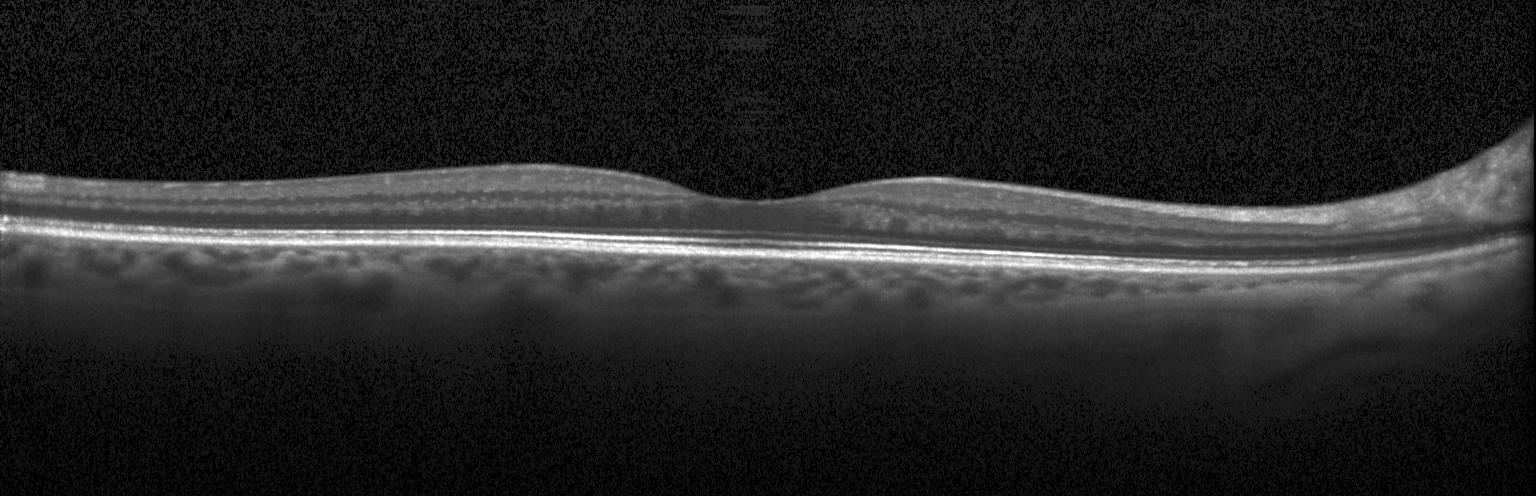

OCT B-scan showing no evidence of choroidal neovascularization, diabetic macular edema, or drusen.